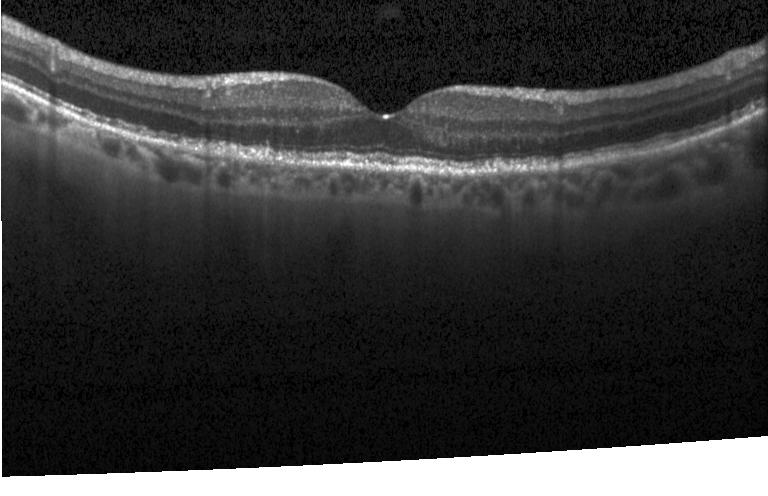 Heidelberg Spectralis; optical coherence tomography scan. Assessment: sub-RPE drusenoid deposits.